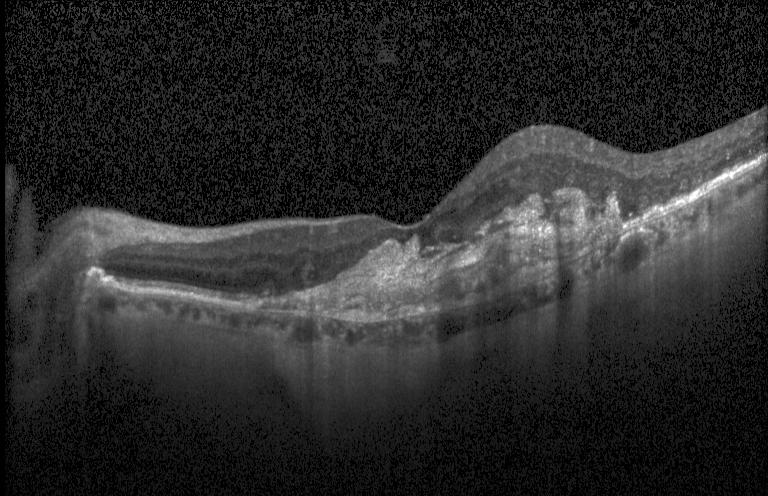

Optical coherence tomography scan
Macular OCT: CNV.